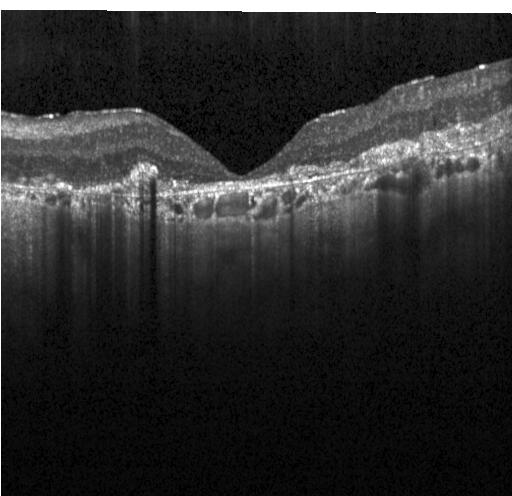 OCT line scan · through the macula.
This B-scan demonstrates choroidal neovascularization.